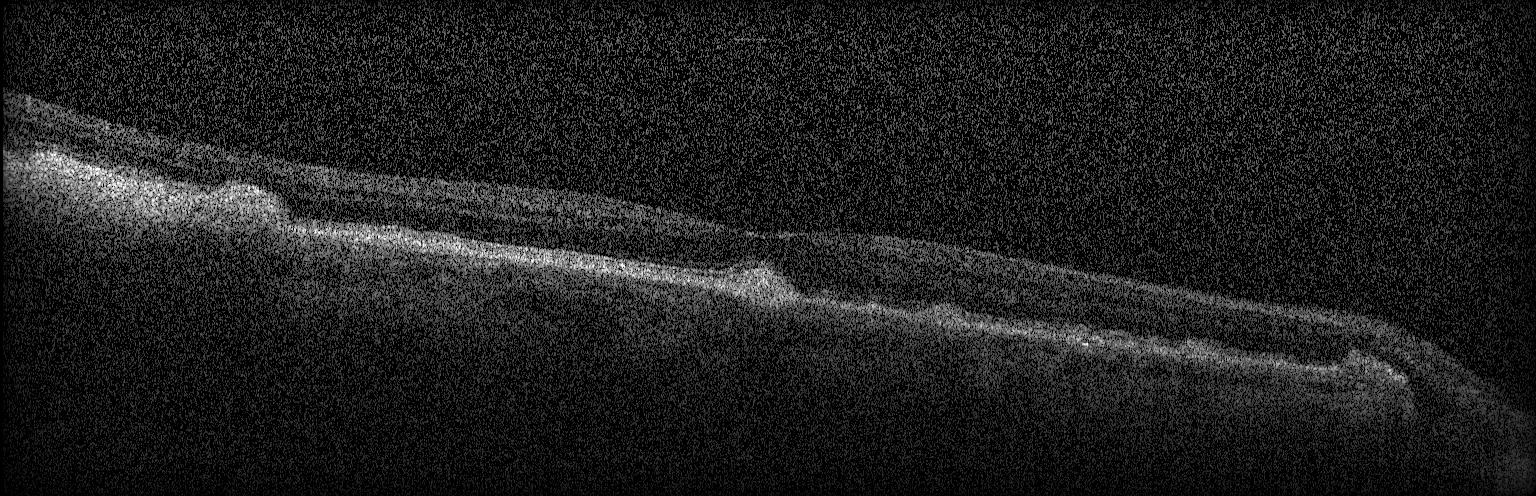 Optical coherence tomography B-scan; macular scan; SD-OCT; instrument: Heidelberg Spectralis — Drusen.